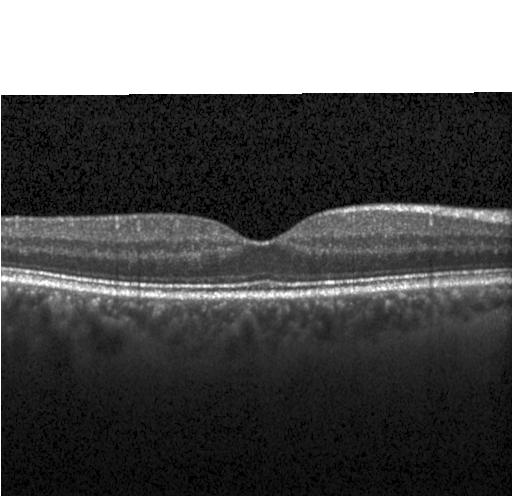 Optical coherence tomography scan; acquired on a Heidelberg Spectralis; SD-OCT — Finding: no CNV, no DME, and no drusen.